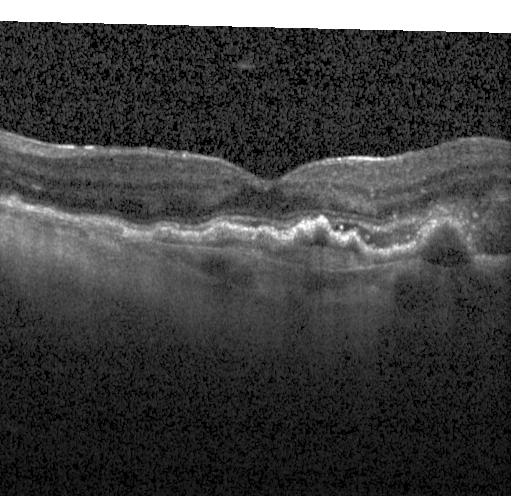

Choroidal neovascularization (CNV).